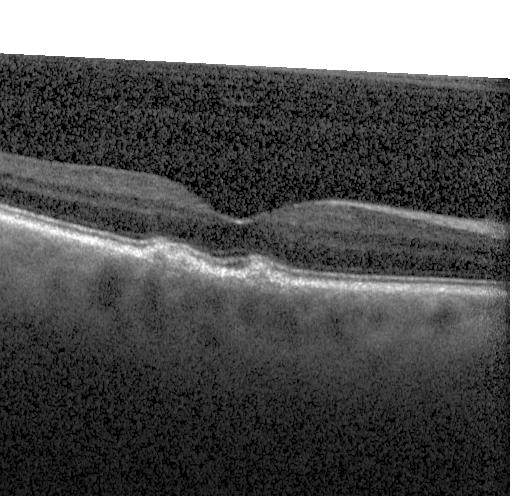

Spectral-domain OCT B-scan: drusen.